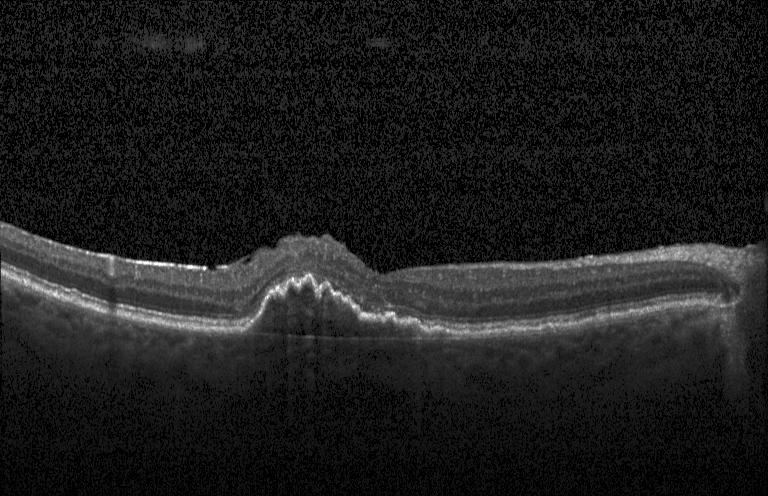 Impression: a choroidal neovascular membrane.